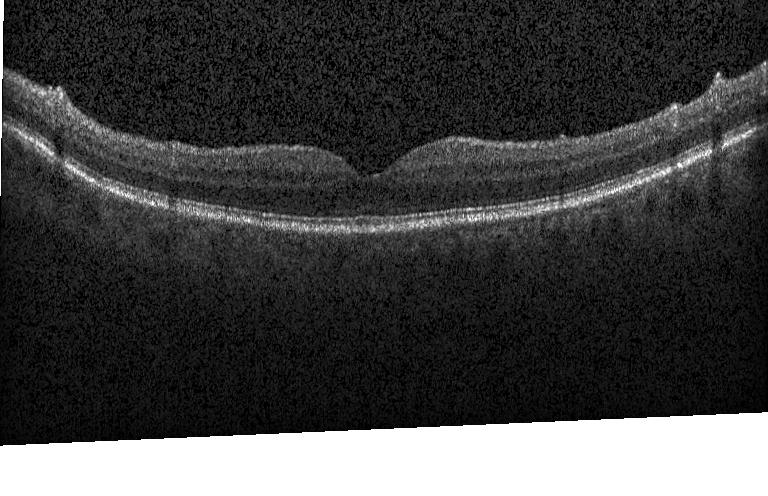

Fovea-centered, OCT B-scan.
Diagnosis: neither choroidal neovascularization, diabetic macular edema, nor drusen.